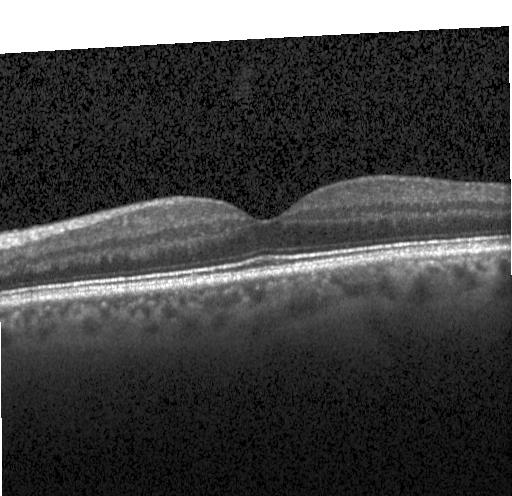 Retinal OCT B-scan.
Macular OCT: no CNV, no DME, and no drusen.